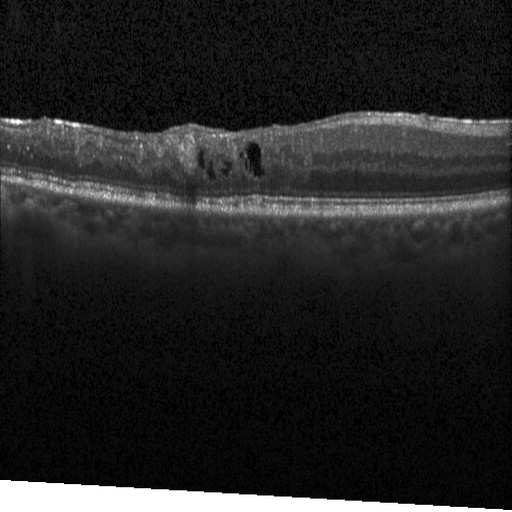

Impression: diabetic macular edema (DME).